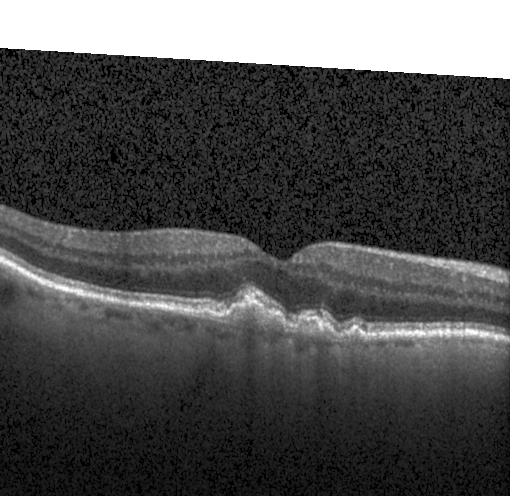
Horizontal scan through the fovea, retinal OCT B-scan, instrument: Heidelberg Spectralis, spectral-domain OCT. Macular OCT: sub-RPE drusenoid deposits.